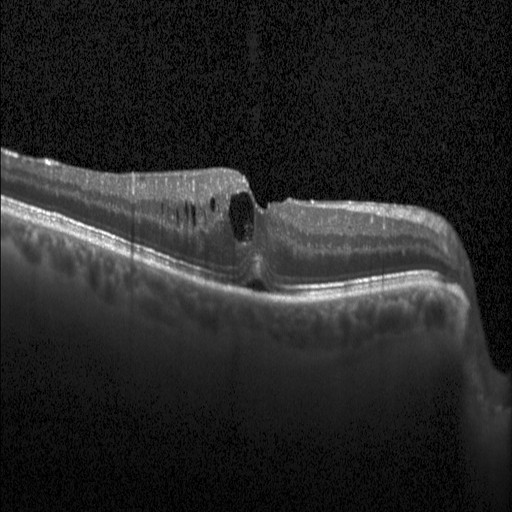

Macular OCT demonstrating diabetic macular edema.